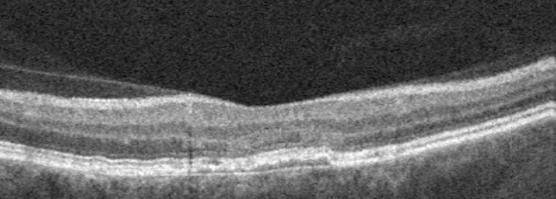
Diagnosis: AMD.